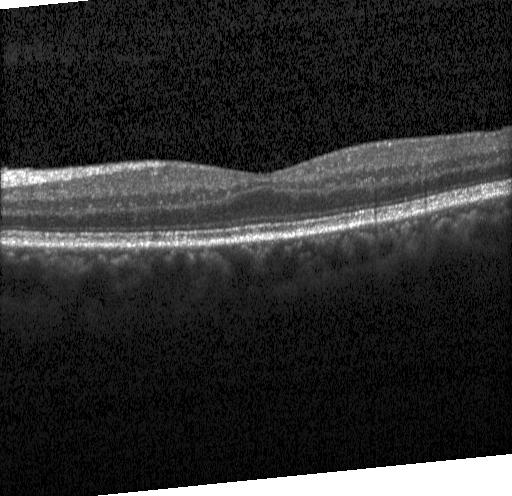
Acquired on a Heidelberg Spectralis, optical coherence tomography B-scan
Diagnosis: no choroidal neovascularization, no diabetic macular edema, and no drusen.